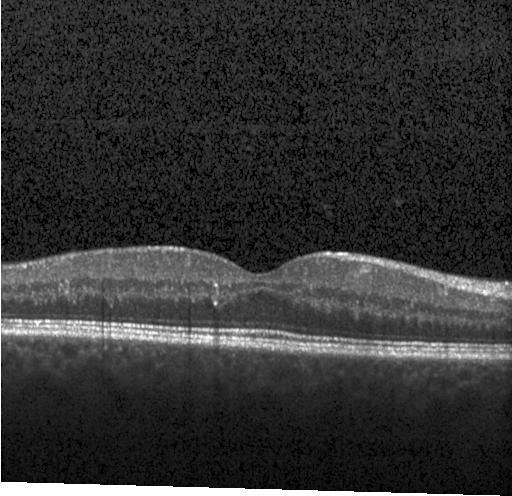

Finding: no evidence of choroidal neovascularization, diabetic macular edema, or drusen.